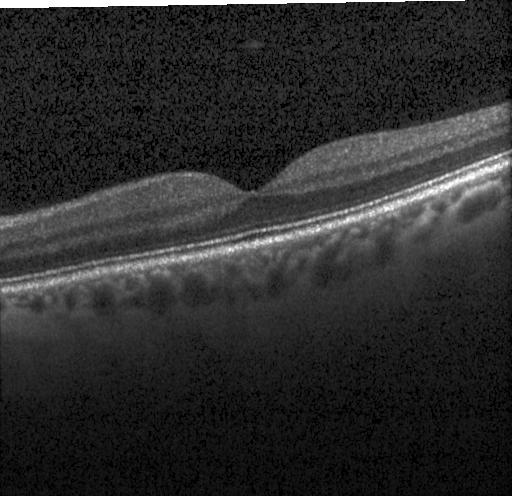
Spectral-domain OCT B-scan: no evidence of choroidal neovascularization, diabetic macular edema, or drusen.